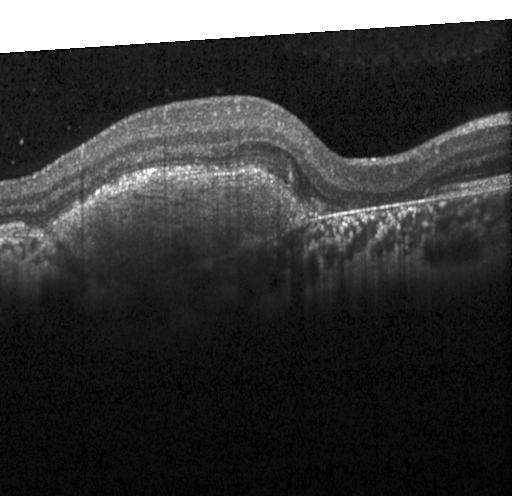
A choroidal neovascular membrane.